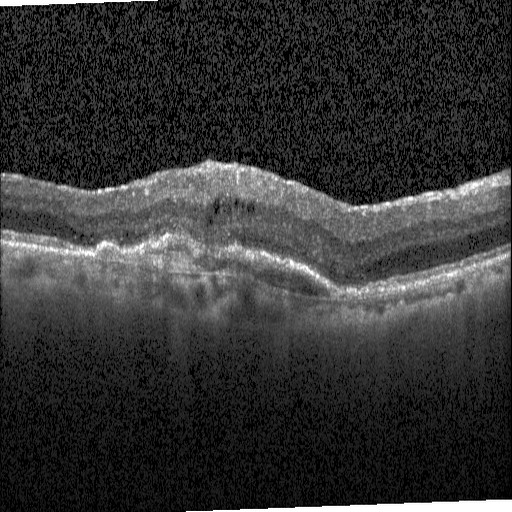 Impression: diabetic macular edema (DME).